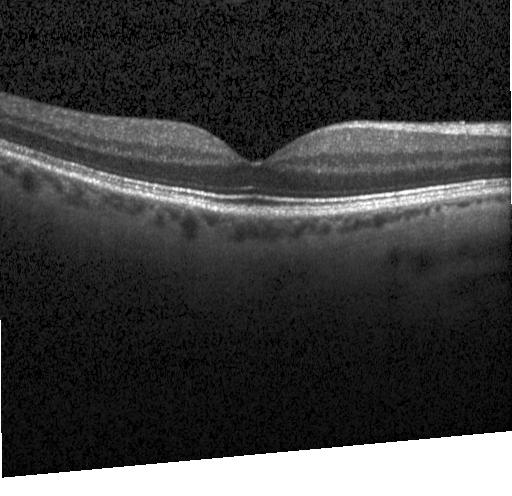

Diagnosis: neither CNV, DME, nor drusen.